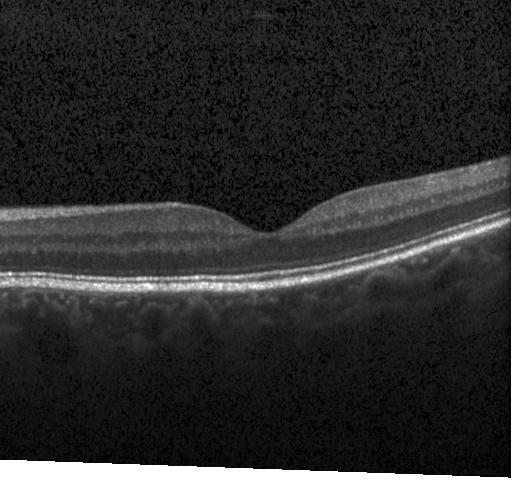 Macular OCT: neither CNV, DME, nor drusen.